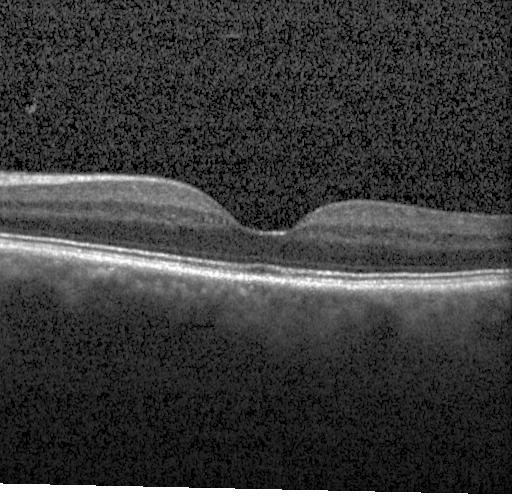
Macular OCT: no choroidal neovascularization, diabetic macular edema, or drusen.